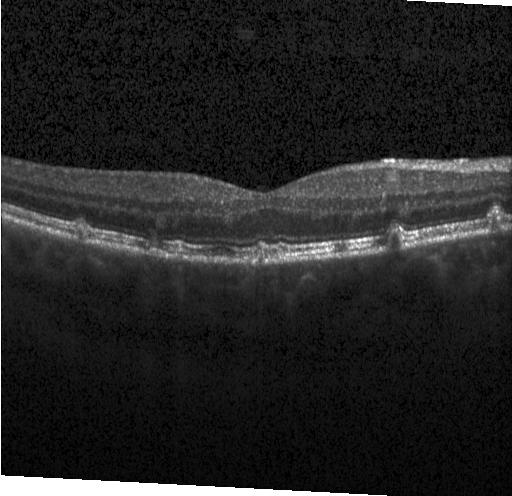 Optical coherence tomography B-scan
Dx: sub-RPE drusenoid deposits.